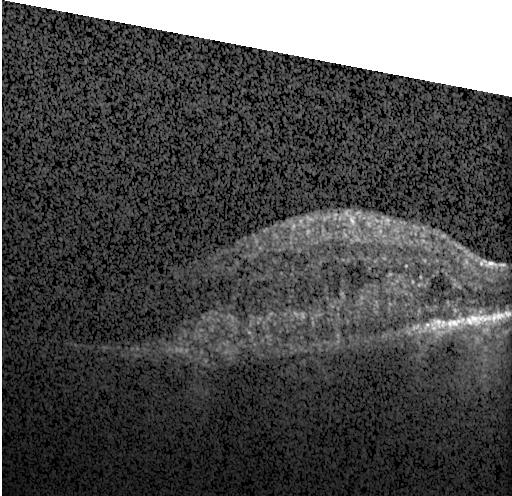

Heidelberg Spectralis OCT system · retinal OCT cross-section · spectral-domain optical coherence tomography. Dx: choroidal neovascularization.